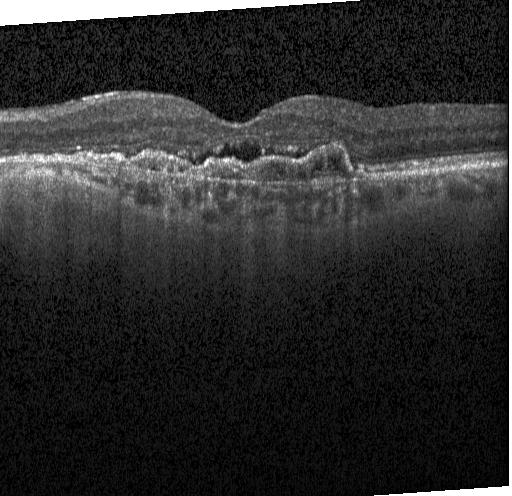
Retinal OCT cross-section. This B-scan demonstrates a choroidal neovascular membrane.